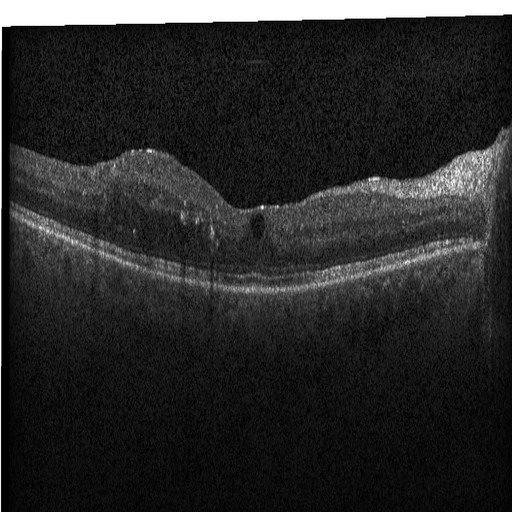 Impression: diabetic macular edema.